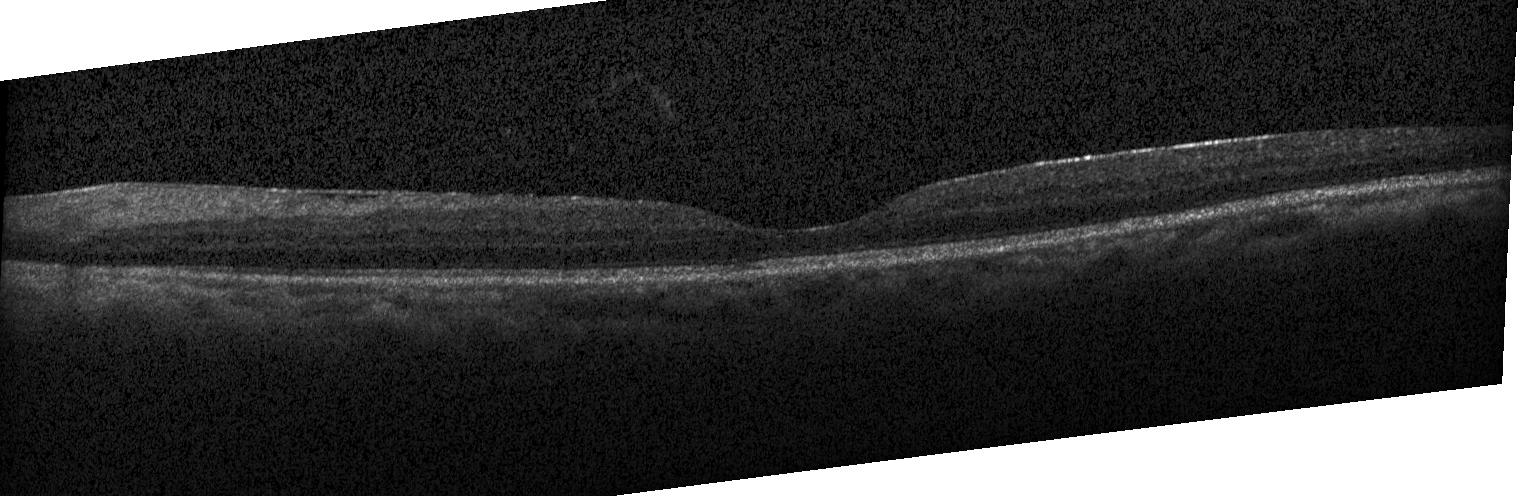
OCT B-scan · horizontal scan through the fovea · Heidelberg Spectralis · spectral-domain OCT. Diagnosis: no choroidal neovascularization, no diabetic macular edema, and no drusen.